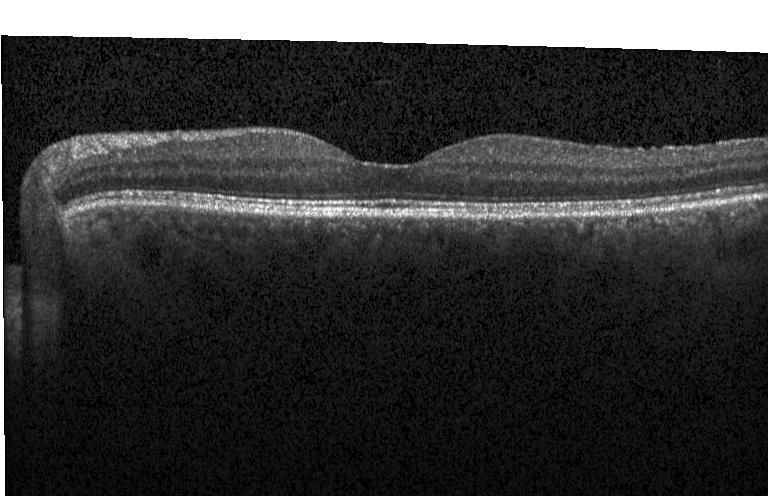 Assessment: no choroidal neovascularization, no diabetic macular edema, and no drusen.